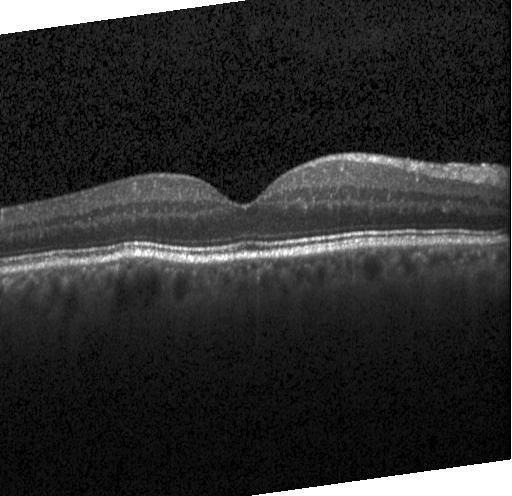

OCT finding: neither choroidal neovascularization, diabetic macular edema, nor drusen.